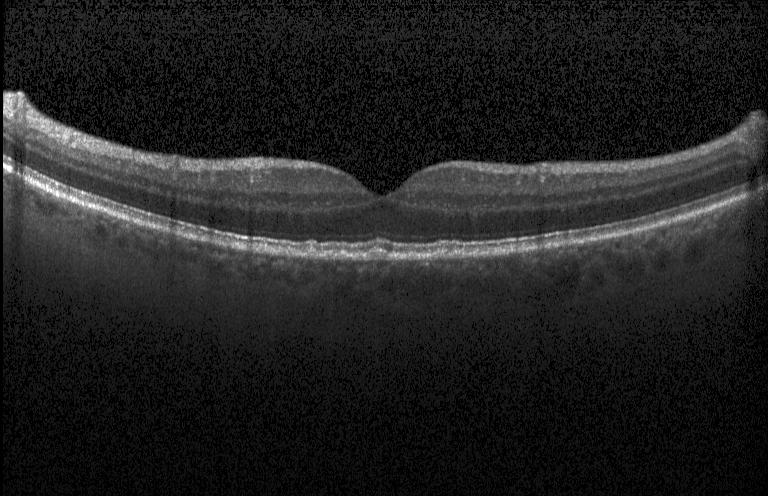
OCT line scan. The scan shows drusen.